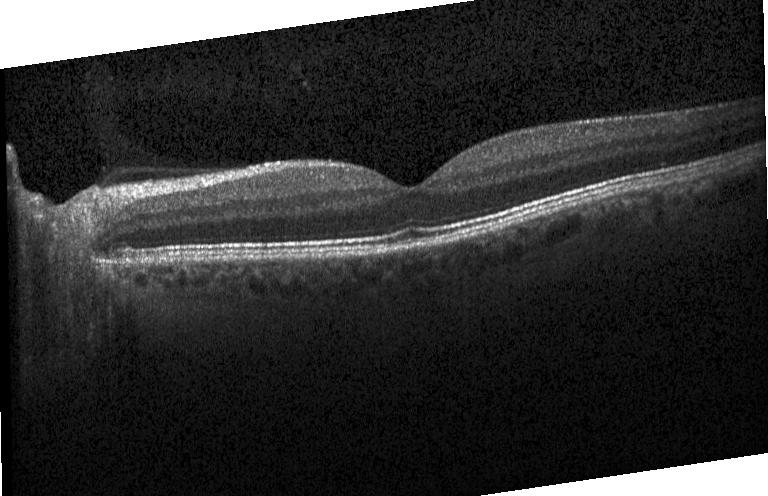 Optical coherence tomography B-scan
Macular OCT: no evidence of choroidal neovascularization, diabetic macular edema, or drusen.